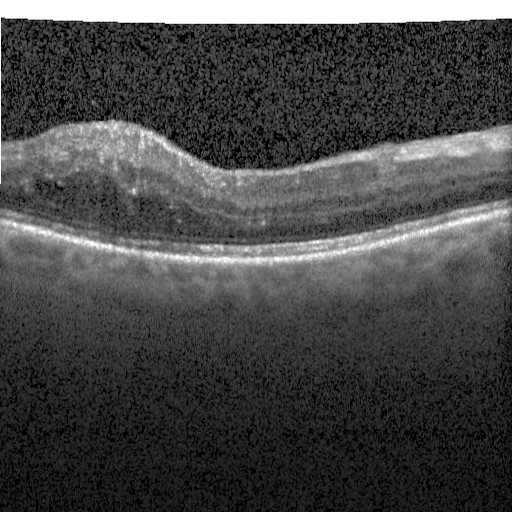
The scan shows DME.